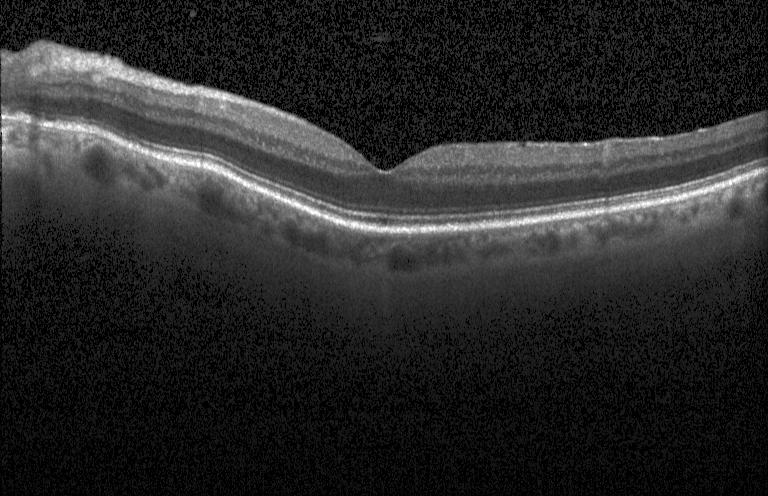
No choroidal neovascularization, no diabetic macular edema, and no drusen.